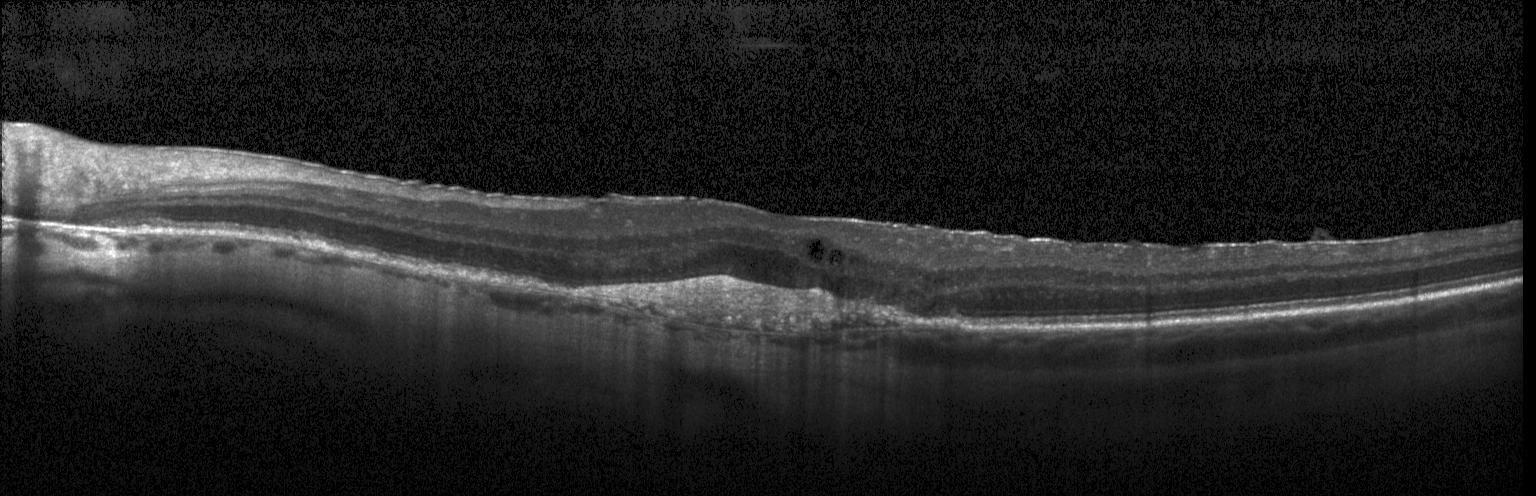 Spectral-domain optical coherence tomography; centered on the fovea; optical coherence tomography B-scan; Heidelberg Spectralis OCT system. Finding: choroidal neovascularization.